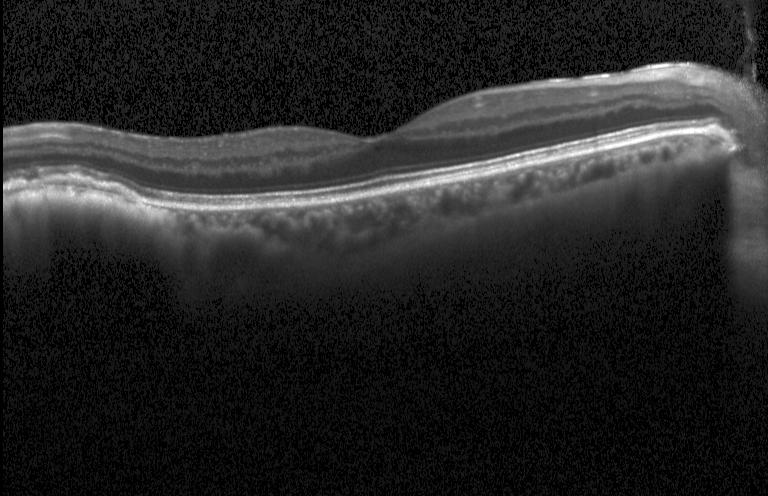

Retinal OCT cross-section showing choroidal neovascularization (CNV).